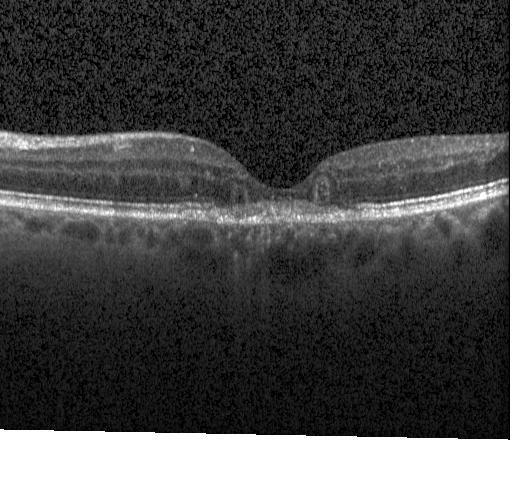 Macular OCT demonstrating a choroidal neovascular membrane.